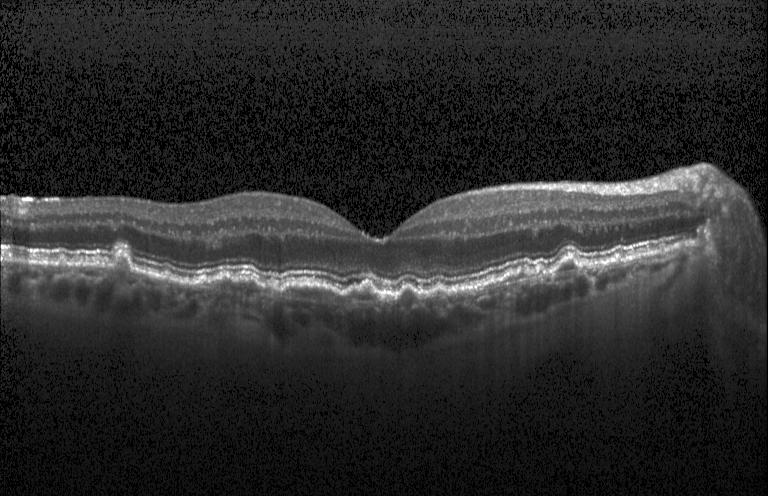

Retinal OCT B-scan, macular scan, spectral-domain optical coherence tomography, acquired on a Heidelberg Spectralis — Finding: drusen.